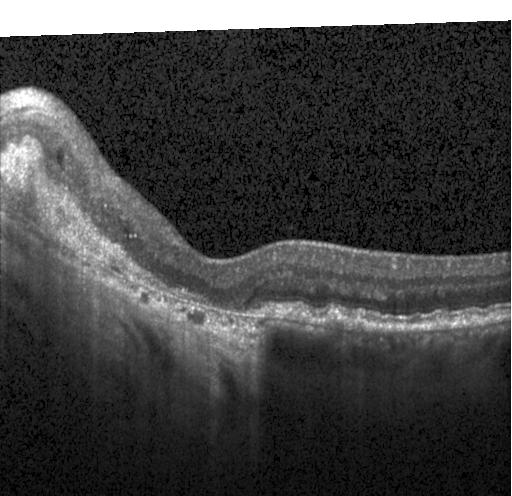

Diagnosis: a choroidal neovascular membrane.